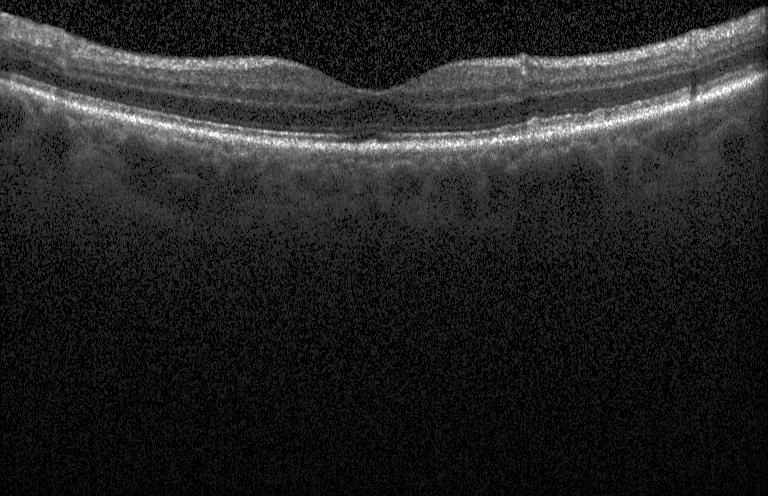
Spectral-domain OCT B-scan: no CNV, no DME, and no drusen.